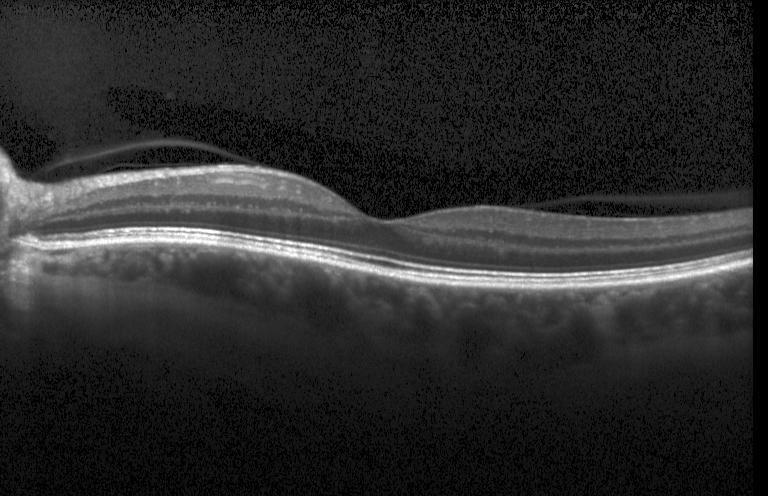 Impression: no choroidal neovascularization, no diabetic macular edema, and no drusen.